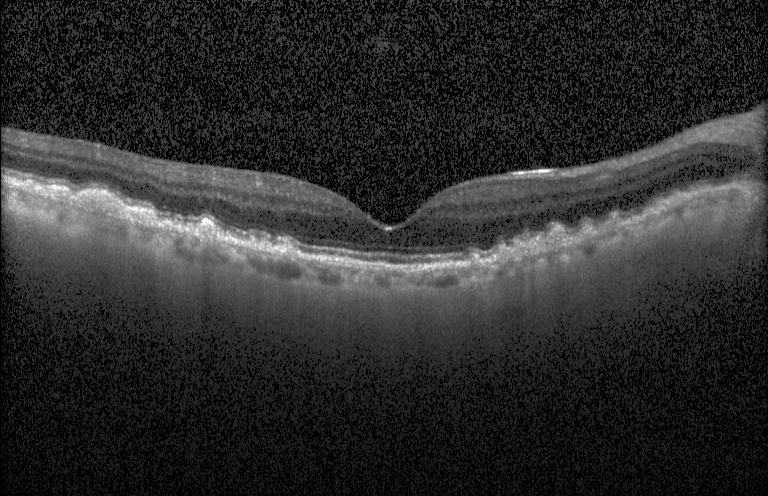 Horizontal scan through the fovea, retinal OCT B-scan, instrument: Heidelberg Spectralis, spectral-domain OCT. Assessment: multiple drusen.